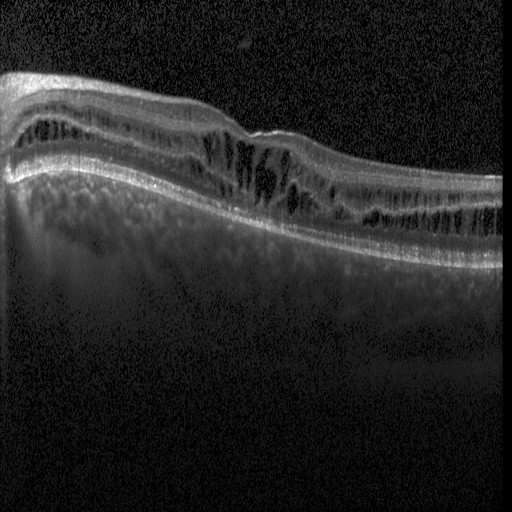 Heidelberg Spectralis · spectral-domain optical coherence tomography · fovea-centered · OCT line scan — Diagnosis: DME.